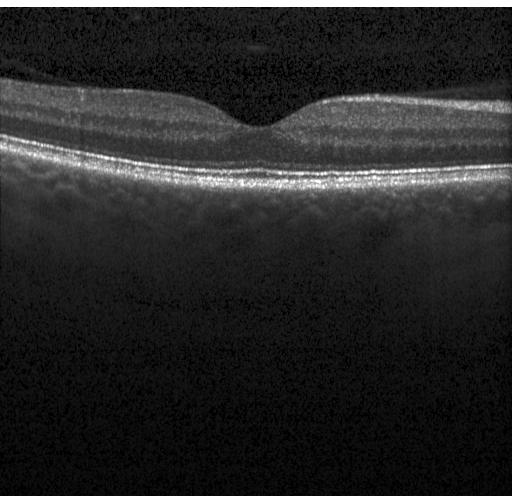
OCT line scan; spectral-domain optical coherence tomography; centered on the fovea
Impression: no evidence of choroidal neovascularization, diabetic macular edema, or drusen.